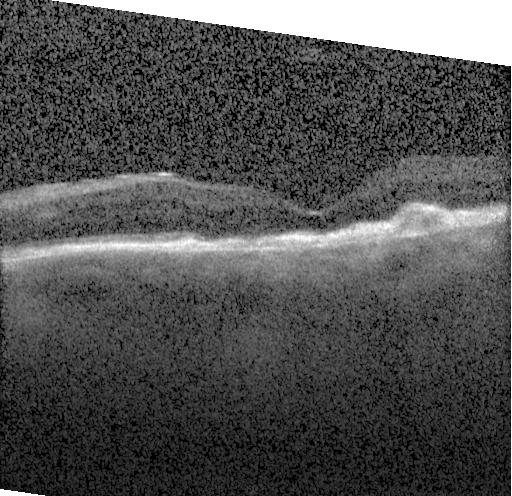 Assessment: a choroidal neovascular membrane.